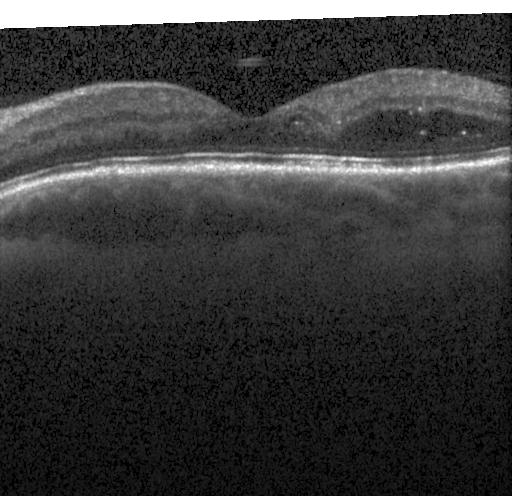
OCT finding: diabetic macular edema (DME).